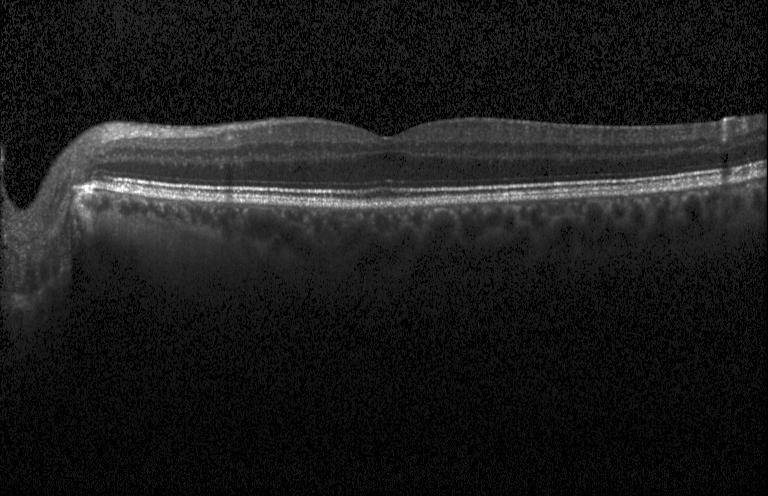

OCT B-scan. Through the macula. Heidelberg Spectralis — Macular OCT: no choroidal neovascularization, no diabetic macular edema, and no drusen.